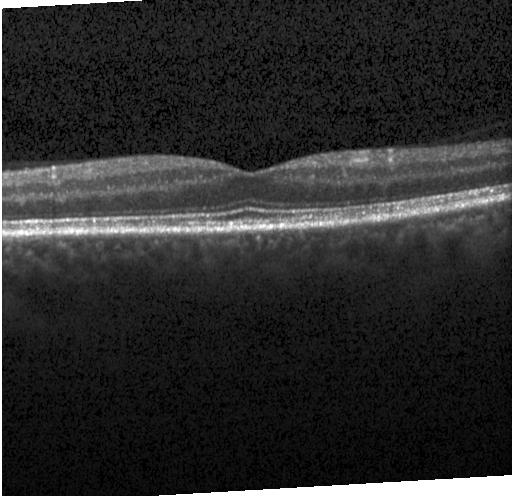

Retinal OCT B-scan · fovea-centered · instrument: Heidelberg Spectralis · SD-OCT. Assessment: no CNV, no DME, and no drusen.